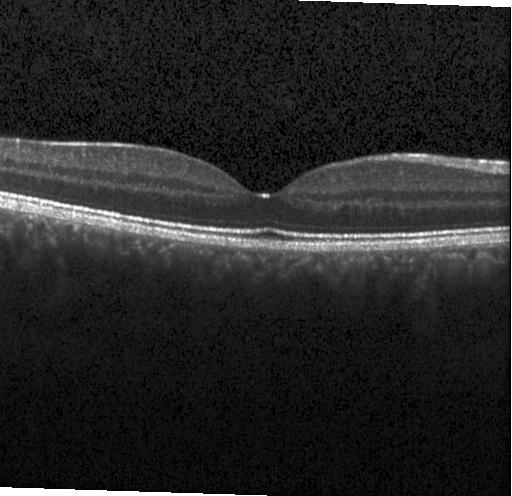
Retinal OCT cross-section; spectral-domain OCT; horizontal scan through the fovea; acquired on a Heidelberg Spectralis
Macular OCT: neither CNV, DME, nor drusen.